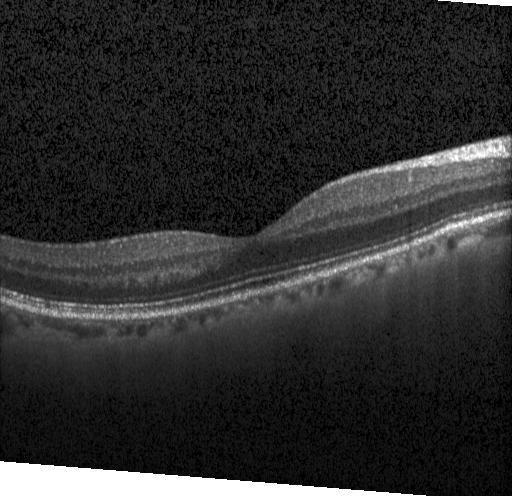

Finding: neither choroidal neovascularization, diabetic macular edema, nor drusen.